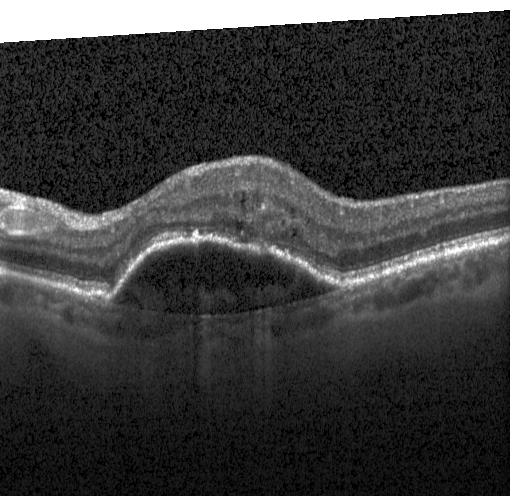

Macular scan · retinal OCT B-scan. Impression: a choroidal neovascular membrane.